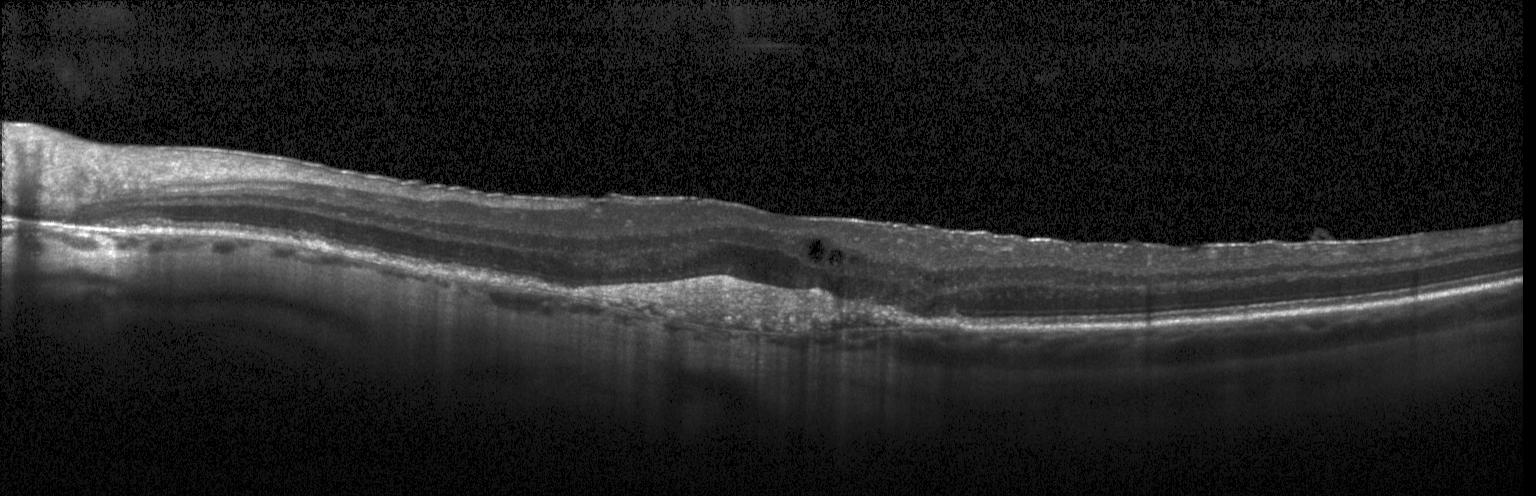
Diagnosis: choroidal neovascularization (CNV).